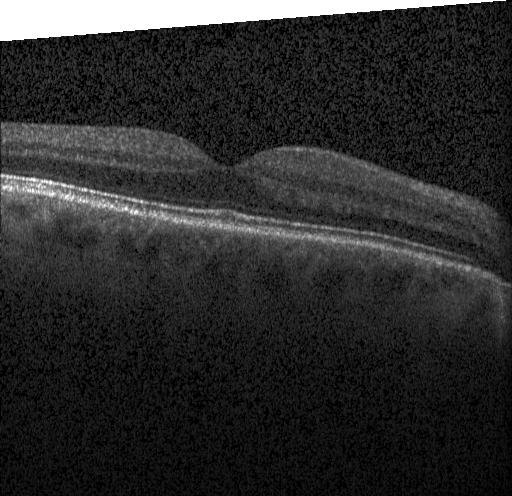
Impression: no evidence of choroidal neovascularization, diabetic macular edema, or drusen.